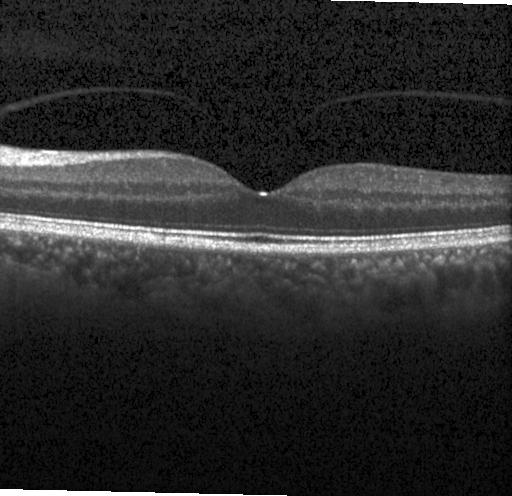
Finding: neither CNV, DME, nor drusen.